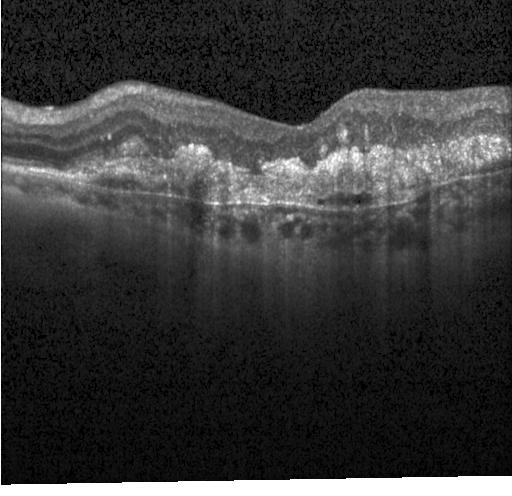
Spectral-domain optical coherence tomography; instrument: Heidelberg Spectralis; through the macula; optical coherence tomography B-scan — Impression: a choroidal neovascular membrane.